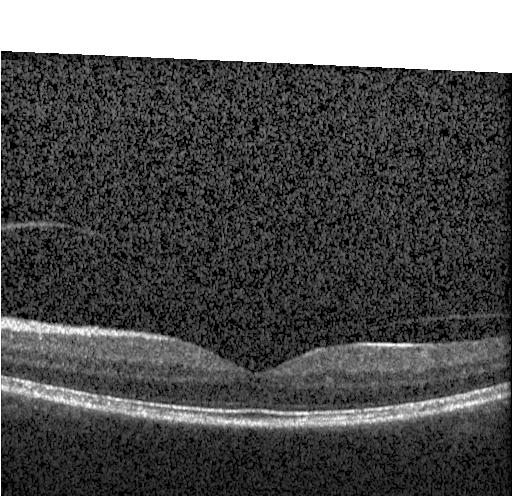

SD-OCT. Heidelberg Spectralis. Retinal OCT cross-section. Macular scan
Impression: no choroidal neovascularization, no diabetic macular edema, and no drusen.